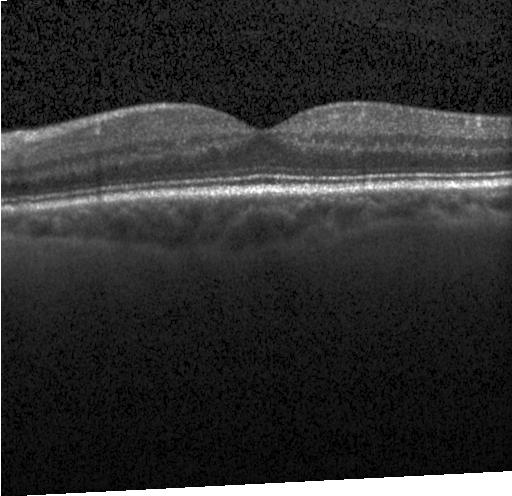 Assessment: neither CNV, DME, nor drusen.